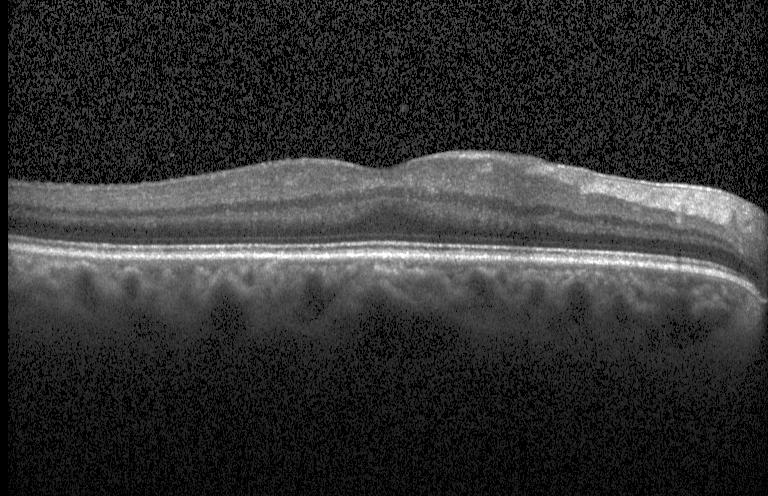

Diagnosis: no evidence of choroidal neovascularization, diabetic macular edema, or drusen.